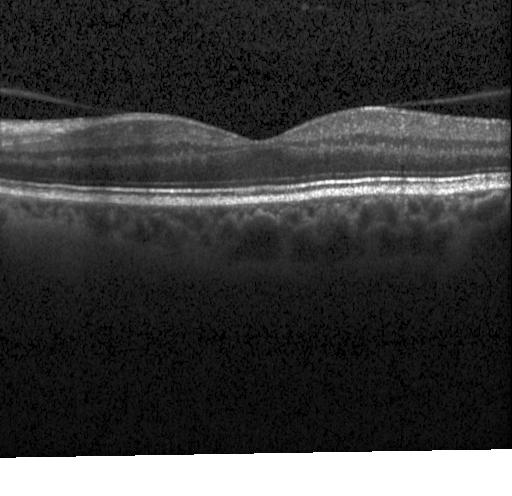
Assessment: no evidence of CNV, DME, or drusen.